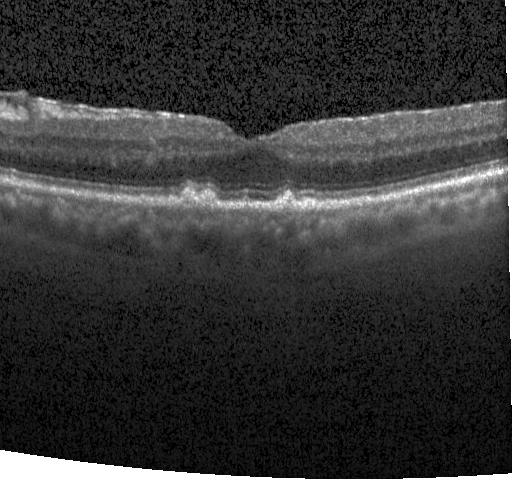 Diagnosis: multiple drusen.